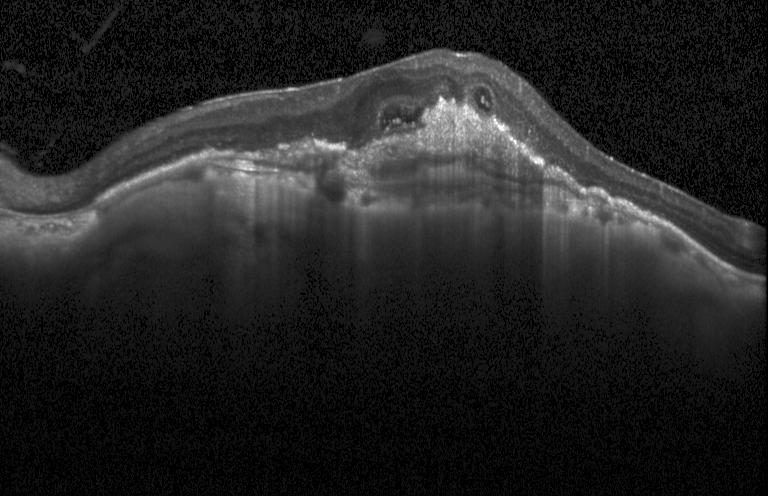

Dx: choroidal neovascularization.